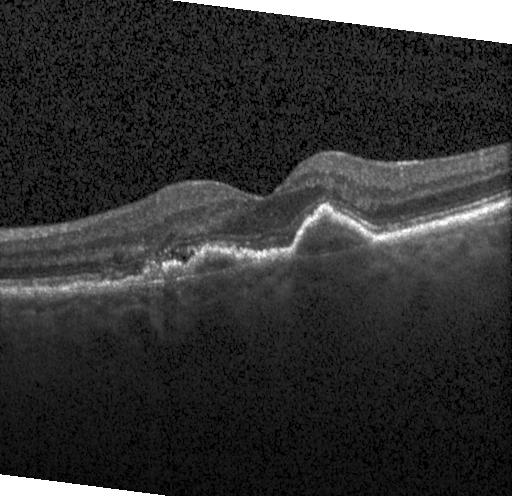

Retinal OCT B-scan · SD-OCT
Dx: a choroidal neovascular membrane.